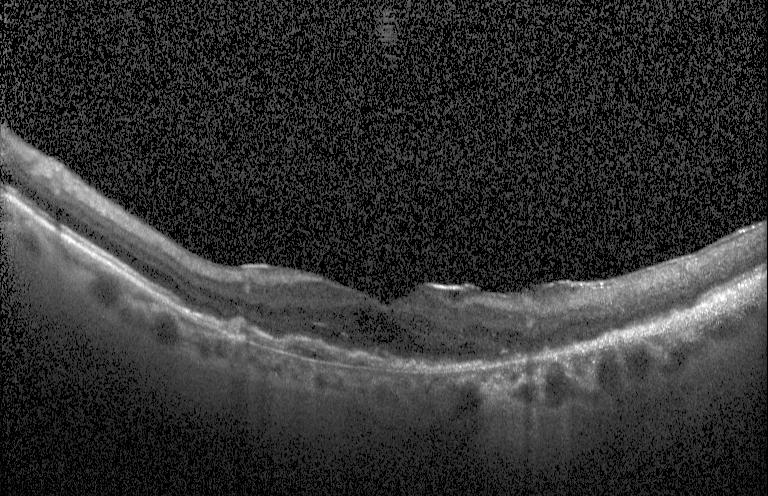 Optical coherence tomography B-scan — Impression: a choroidal neovascular membrane.